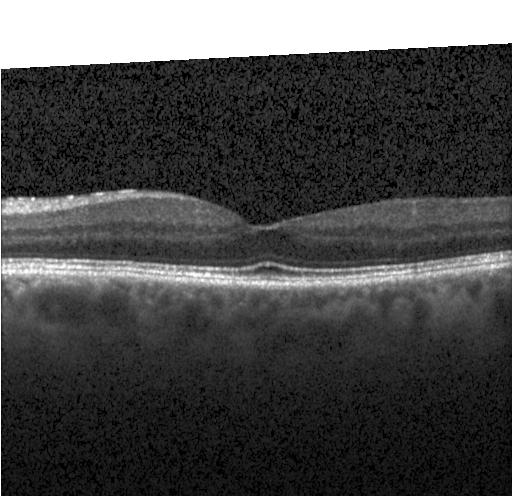 SD-OCT; retinal OCT B-scan
Finding: no evidence of CNV, DME, or drusen.